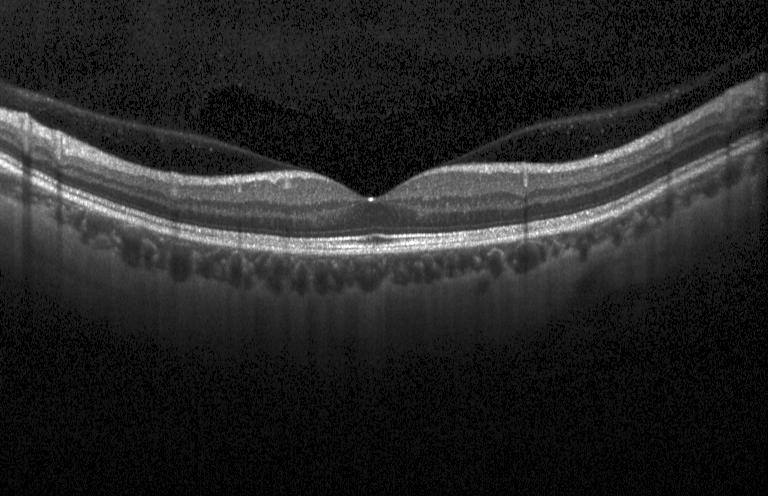
OCT line scan. Finding: neither choroidal neovascularization, diabetic macular edema, nor drusen.